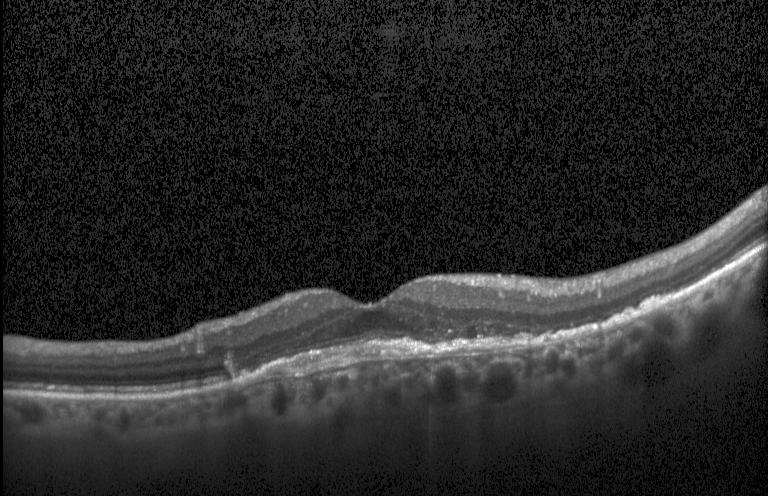 Dx: CNV.